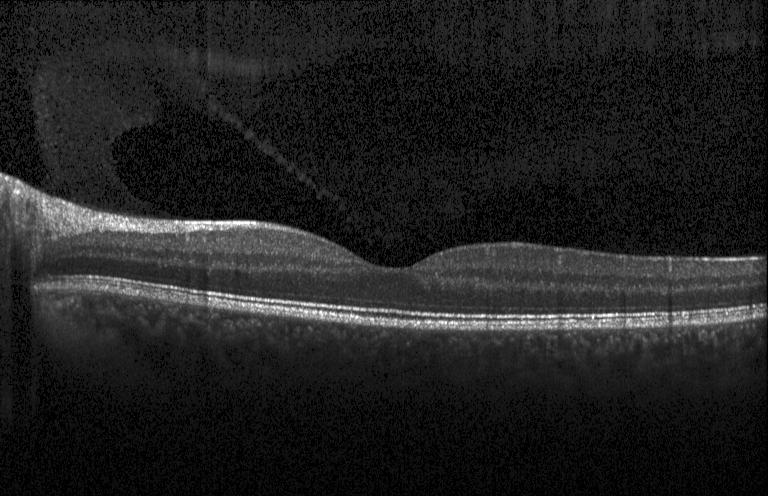 Retinal OCT B-scan. SD-OCT.
Diagnosis: no CNV, no DME, and no drusen.